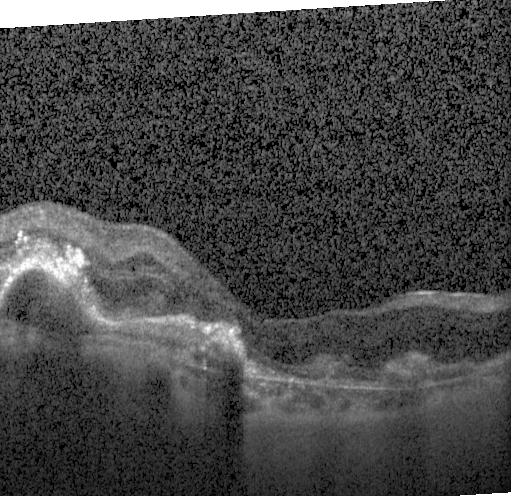 OCT B-scan showing CNV.